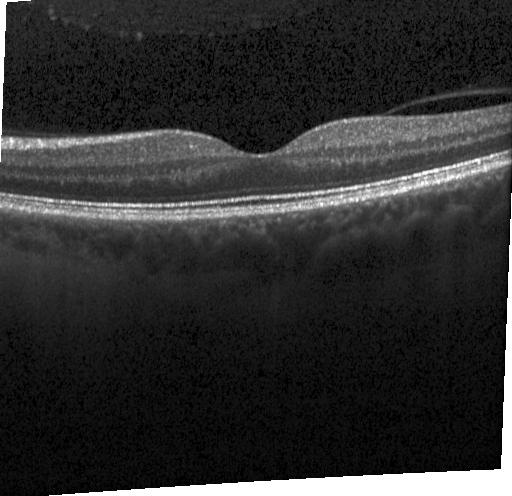

Retinal OCT cross-section showing no choroidal neovascularization, no diabetic macular edema, and no drusen.